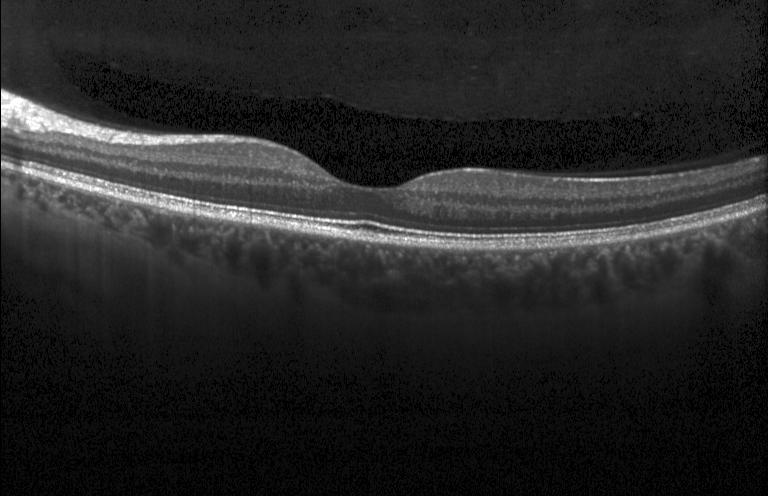 OCT B-scan showing no evidence of choroidal neovascularization, diabetic macular edema, or drusen.